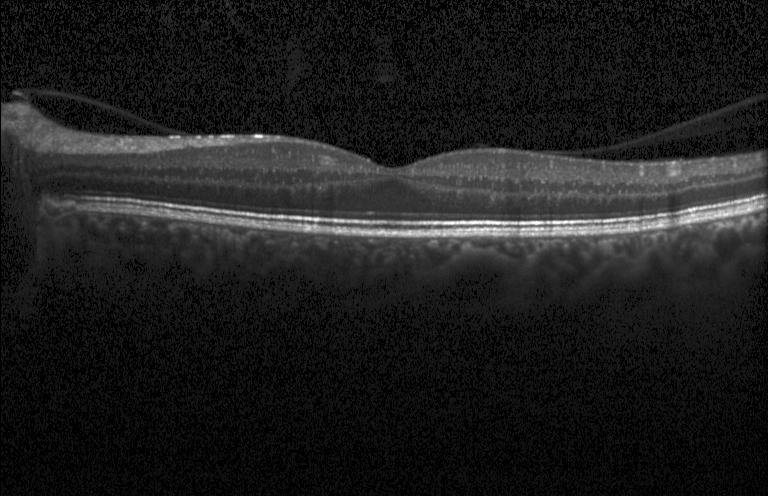

Finding: no CNV, DME, or drusen.